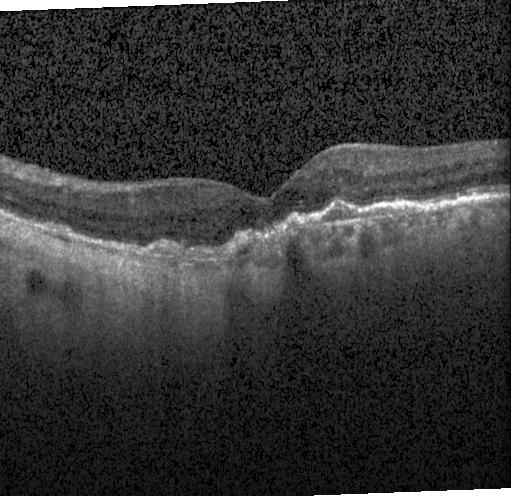

Macular OCT: CNV.